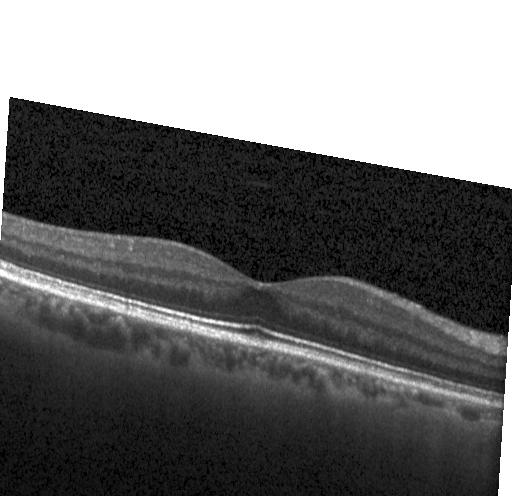 Impression: no evidence of CNV, DME, or drusen.